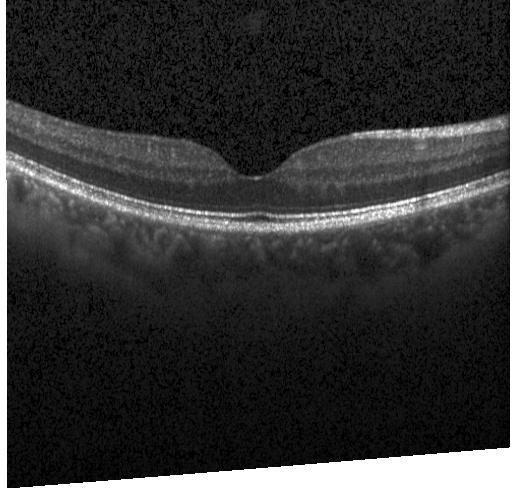
Centered on the fovea; instrument: Heidelberg Spectralis; OCT line scan. This B-scan demonstrates no evidence of CNV, DME, or drusen.